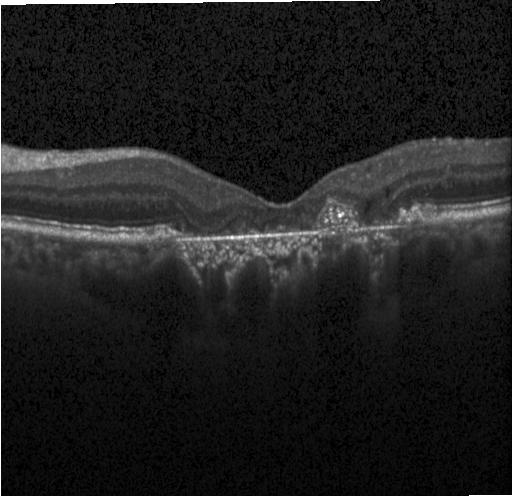 Spectral-domain OCT. Retinal OCT cross-section
Diagnosis: CNV.